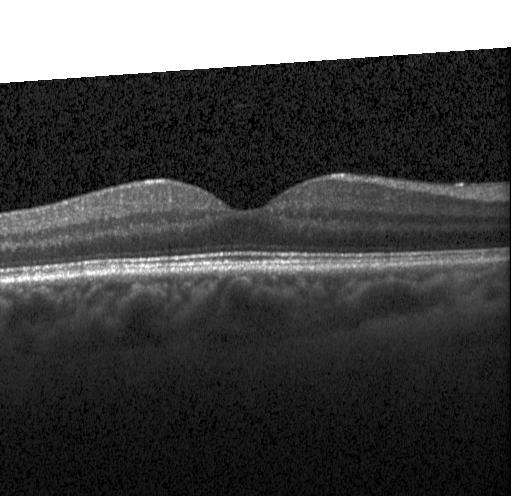

Optical coherence tomography B-scan, spectral-domain optical coherence tomography, fovea-centered.
Neither CNV, DME, nor drusen.